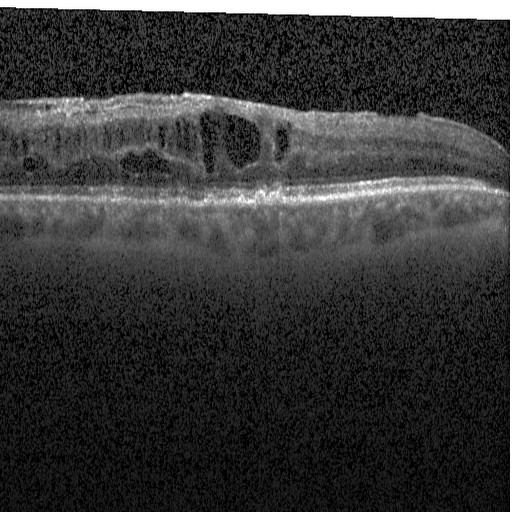 Retinal OCT cross-section
Dx: diabetic macular edema.